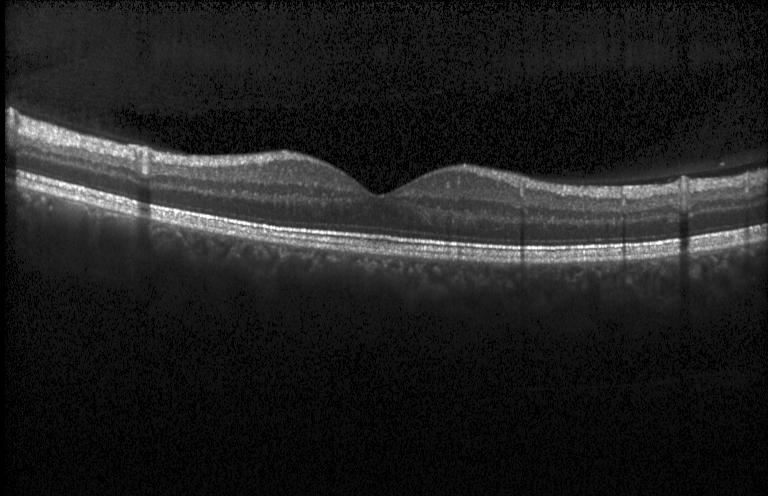 Spectral-domain optical coherence tomography, Heidelberg Spectralis, optical coherence tomography scan, through the macula
Assessment: neither CNV, DME, nor drusen.